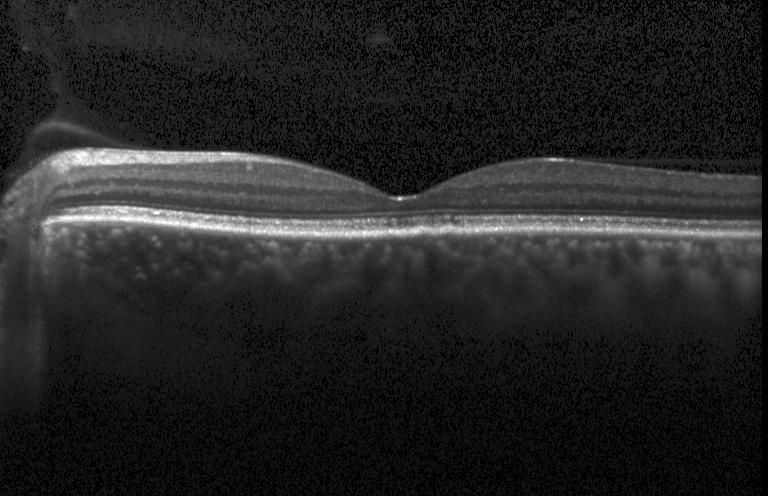 Dx: neither CNV, DME, nor drusen.